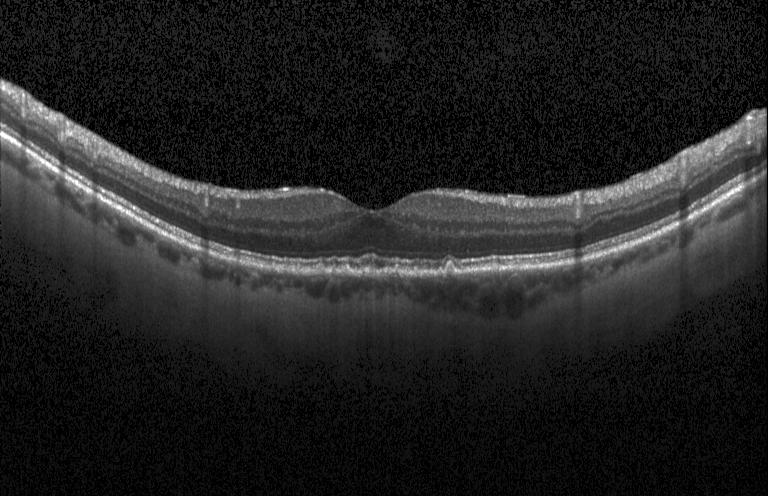
Retinal OCT B-scan, SD-OCT, macular scan.
This B-scan demonstrates multiple drusen.